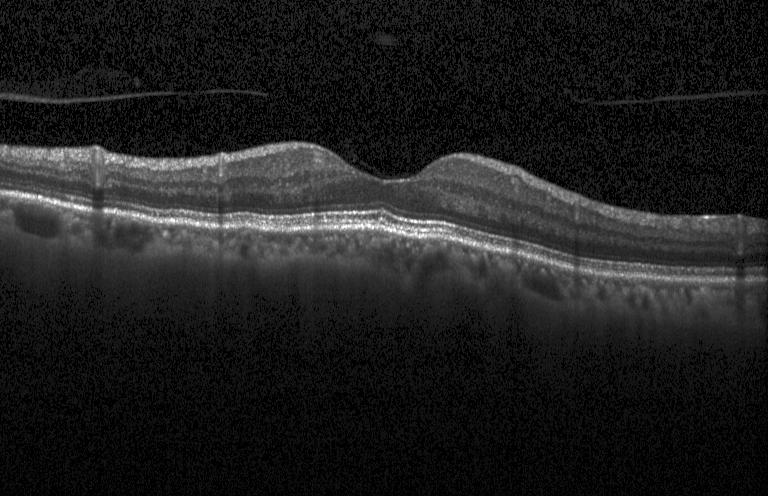
Optical coherence tomography B-scan; centered on the fovea
The scan shows no choroidal neovascularization, diabetic macular edema, or drusen.